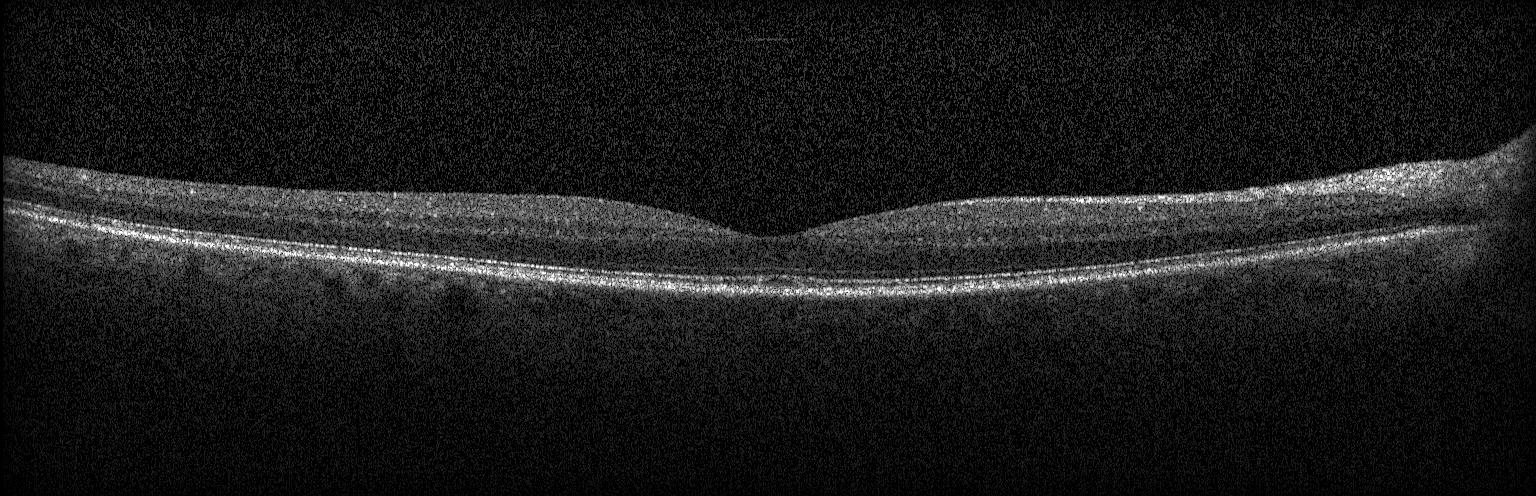

Impression: neither choroidal neovascularization, diabetic macular edema, nor drusen.